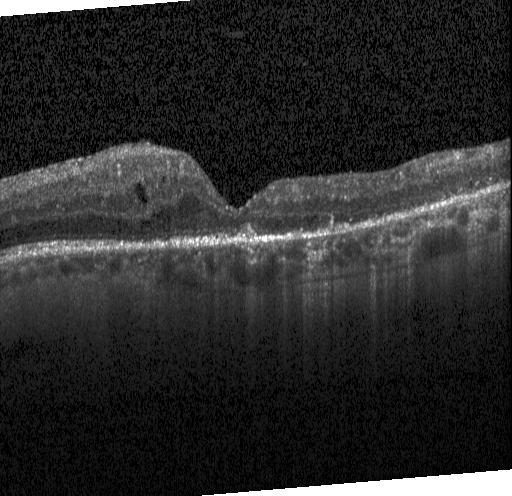
Horizontal scan through the fovea, OCT B-scan. This B-scan demonstrates diabetic macular edema.